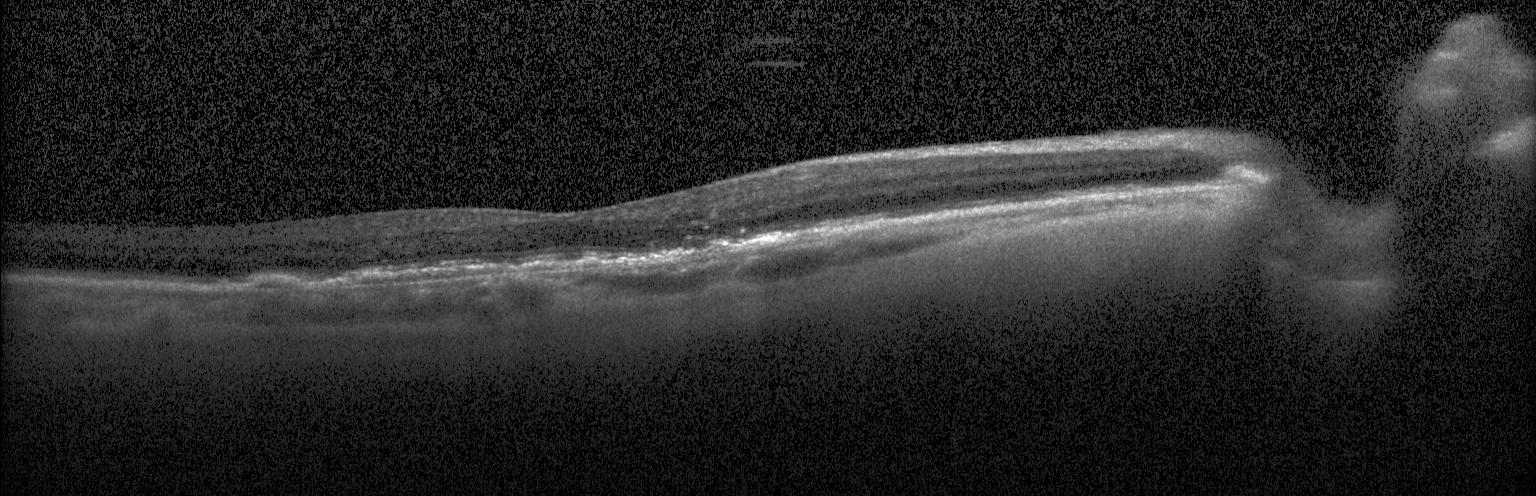 The scan shows a choroidal neovascular membrane.